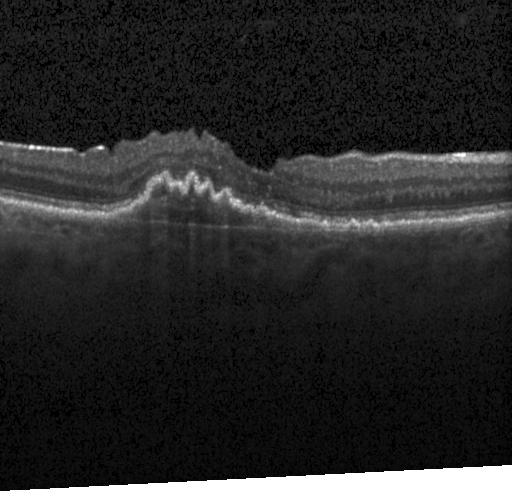
Retinal OCT cross-section · horizontal scan through the fovea — Impression: choroidal neovascularization.